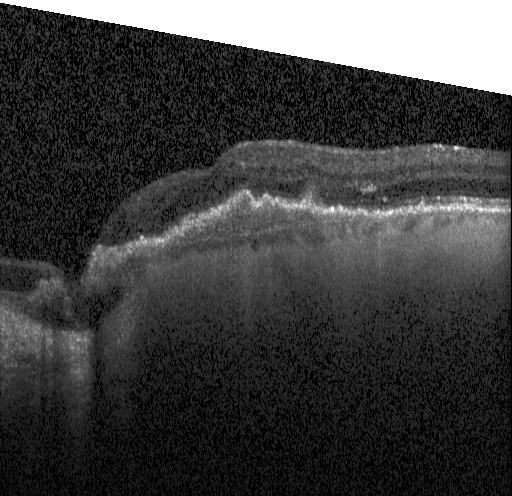
OCT B-scan showing a choroidal neovascular membrane.